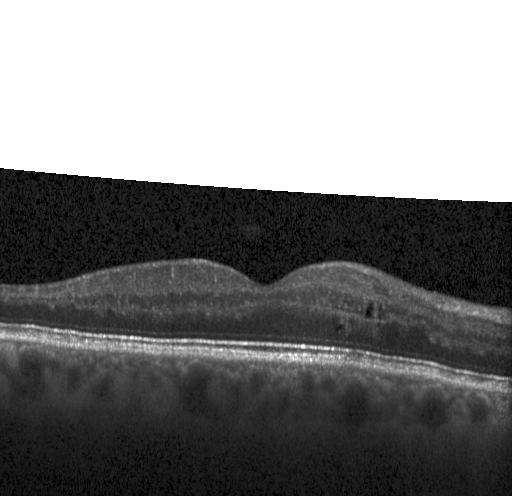 Retinal OCT cross-section; Heidelberg Spectralis; spectral-domain OCT — This B-scan demonstrates diabetic macular edema (DME).